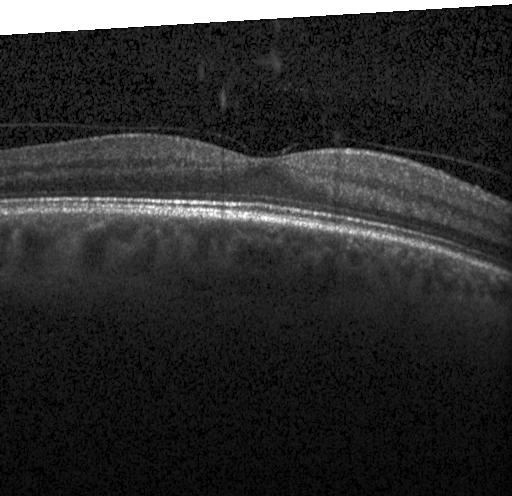

OCT line scan; spectral-domain optical coherence tomography; fovea-centered.
OCT finding: no choroidal neovascularization, diabetic macular edema, or drusen.